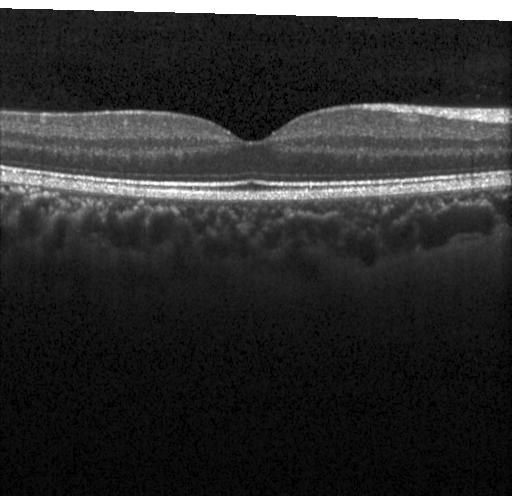 Assessment: no choroidal neovascularization, no diabetic macular edema, and no drusen.